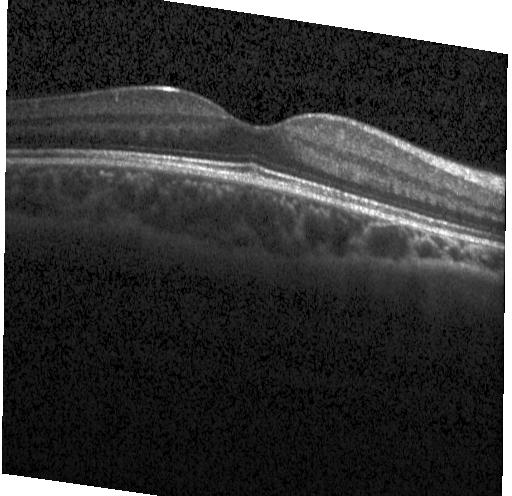

OCT B-scan — Diagnosis: neither CNV, DME, nor drusen.